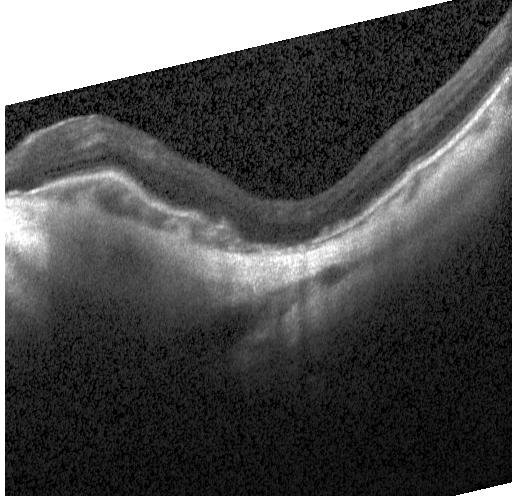 Retinal OCT B-scan. Finding: a choroidal neovascular membrane.